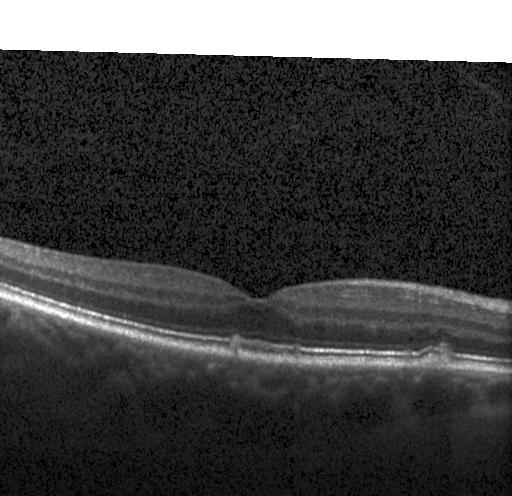 Finding: sub-RPE drusenoid deposits.